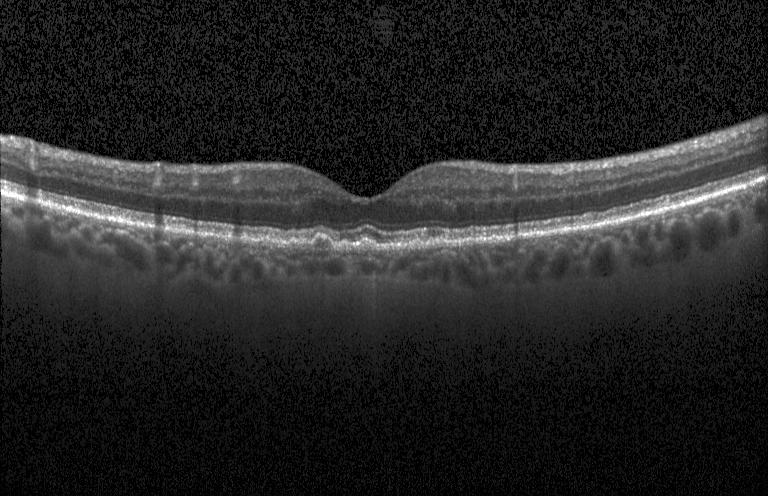 Finding: sub-RPE drusenoid deposits.